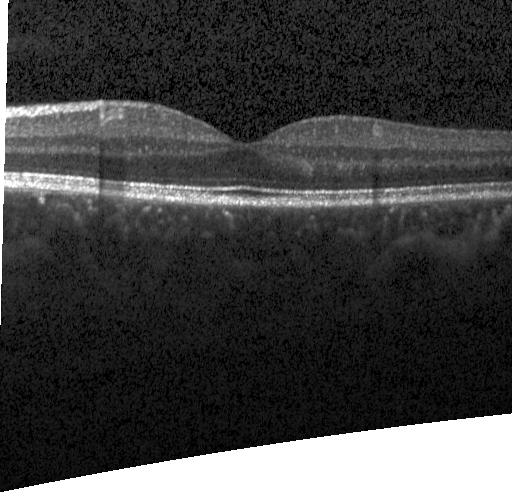

OCT scan showing neither CNV, DME, nor drusen.